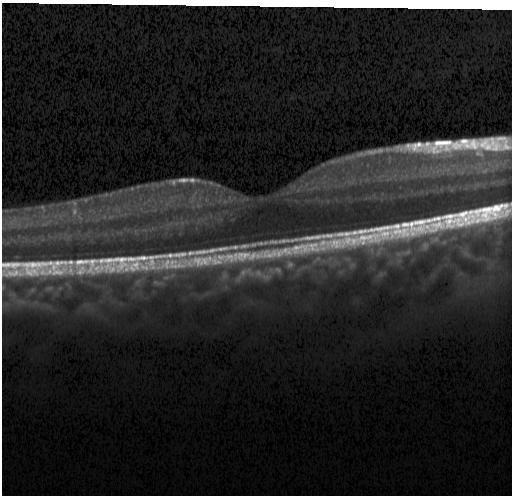

Dx: no evidence of choroidal neovascularization, diabetic macular edema, or drusen.